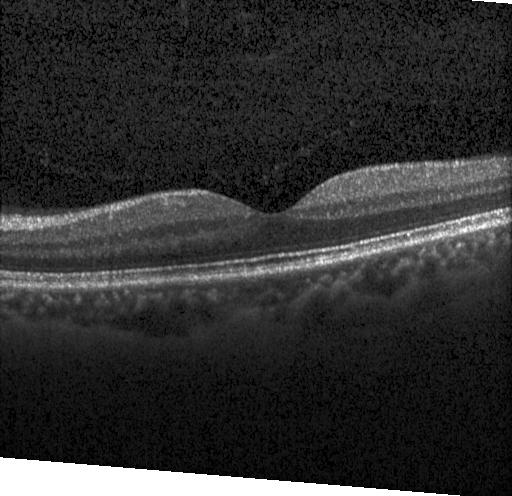 OCT finding: no choroidal neovascularization, diabetic macular edema, or drusen.